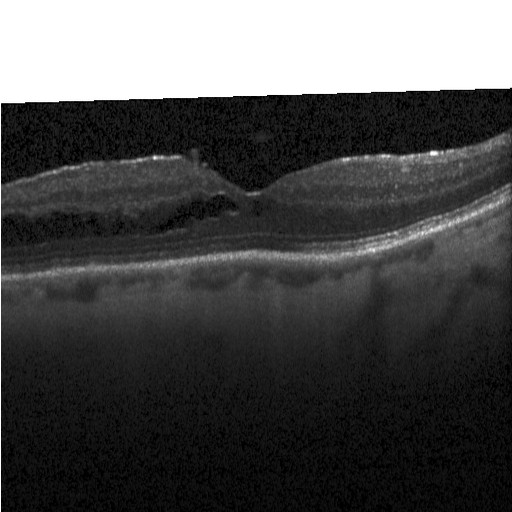

Optical coherence tomography scan
Assessment: diabetic macular edema (DME).